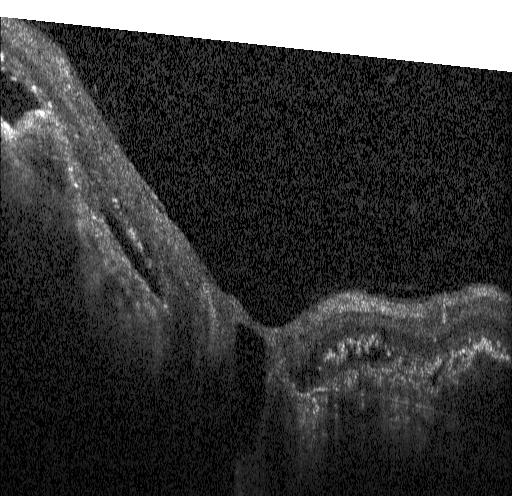
Dx: a choroidal neovascular membrane.